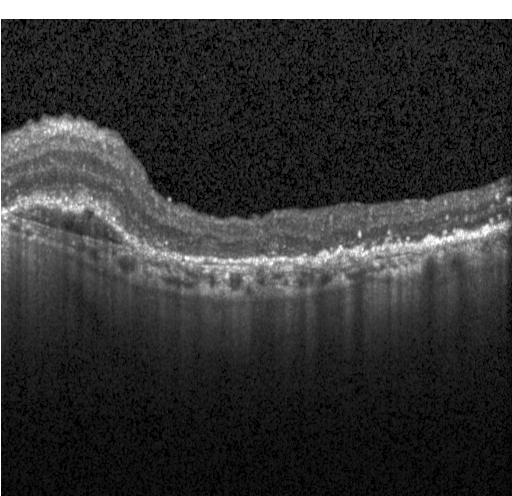
Assessment: a choroidal neovascular membrane.